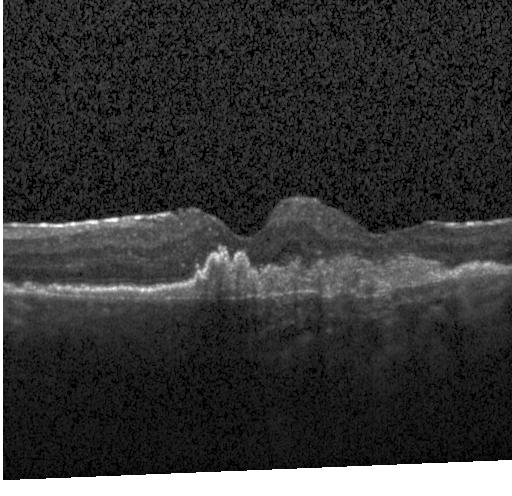

Impression: CNV.